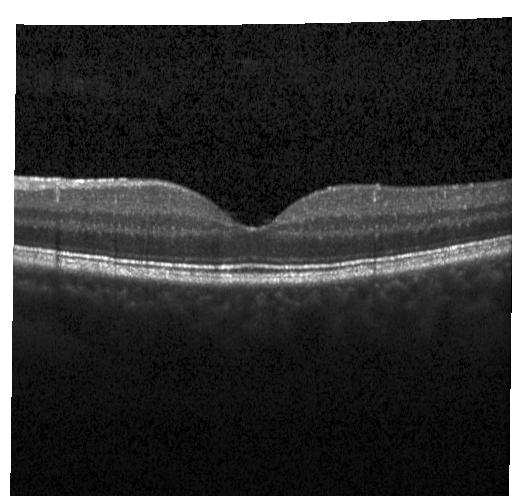 Optical coherence tomography B-scan.
This B-scan demonstrates neither choroidal neovascularization, diabetic macular edema, nor drusen.